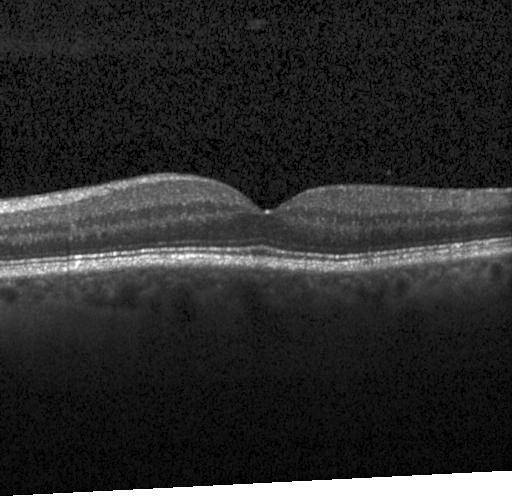
Diagnosis: no choroidal neovascularization, diabetic macular edema, or drusen.